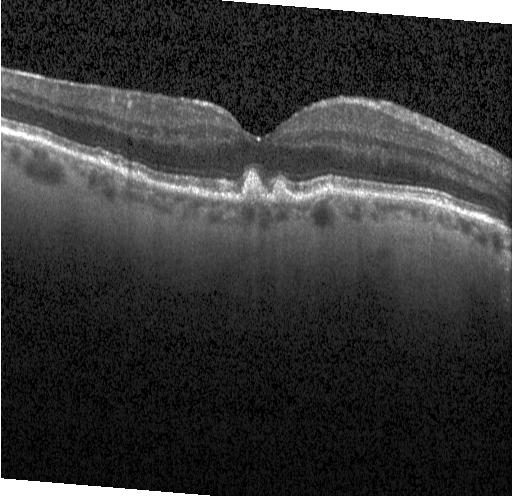 This B-scan demonstrates drusen.